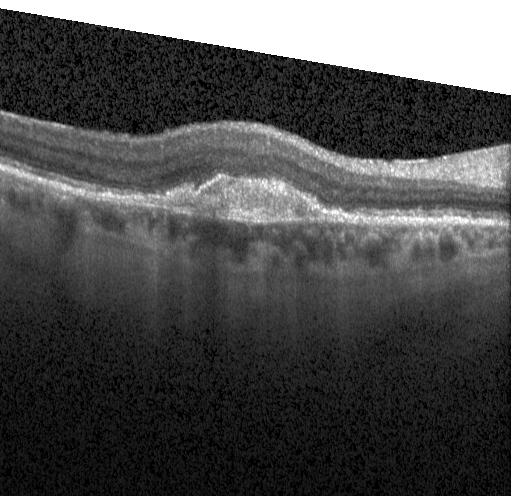
Spectral-domain OCT · Heidelberg Spectralis OCT system · retinal OCT B-scan · horizontal scan through the fovea — Diagnosis: CNV.